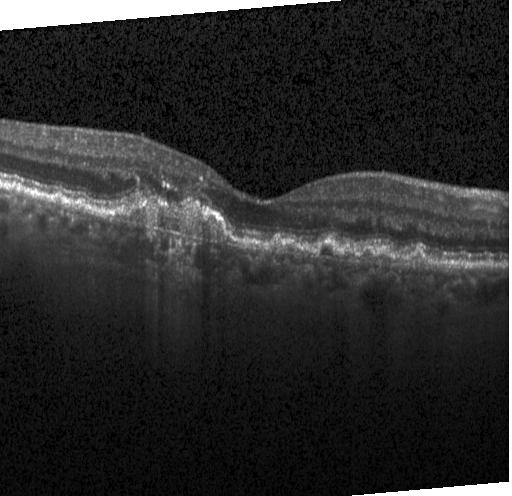 The scan shows a choroidal neovascular membrane.